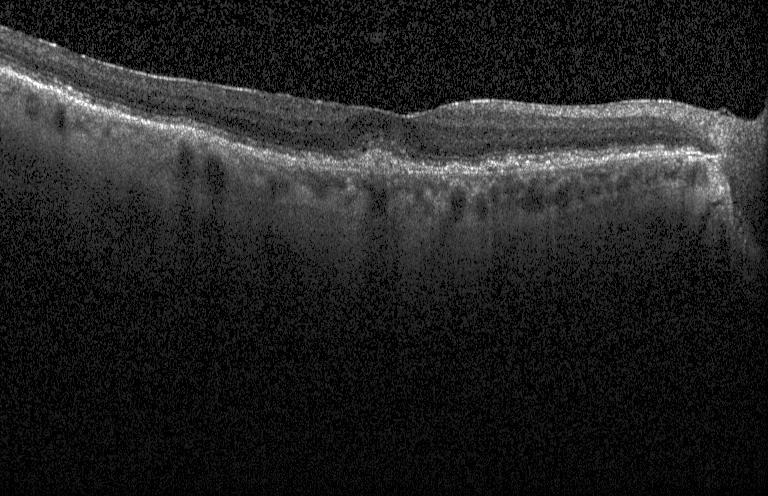
A choroidal neovascular membrane.